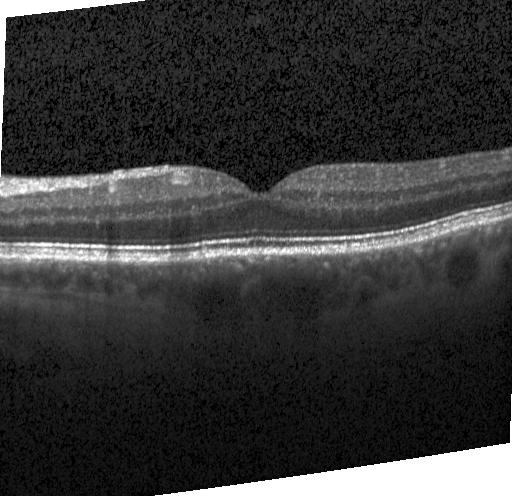 SD-OCT. Heidelberg Spectralis OCT system. Horizontal scan through the fovea. Optical coherence tomography B-scan — Diagnosis: no choroidal neovascularization, diabetic macular edema, or drusen.